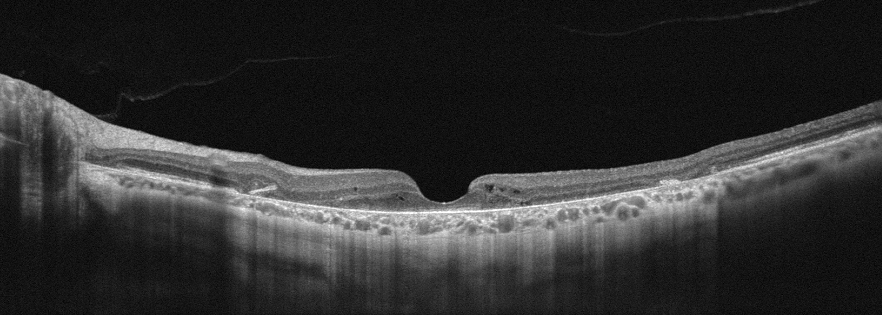 Optical coherence tomography scan — Finding: age-related macular degeneration.